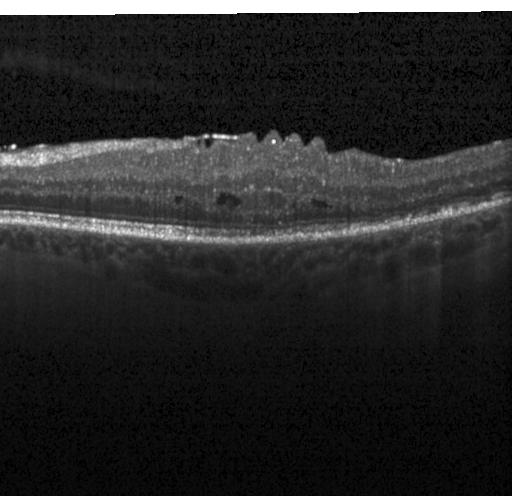

Assessment: diabetic macular edema (DME).